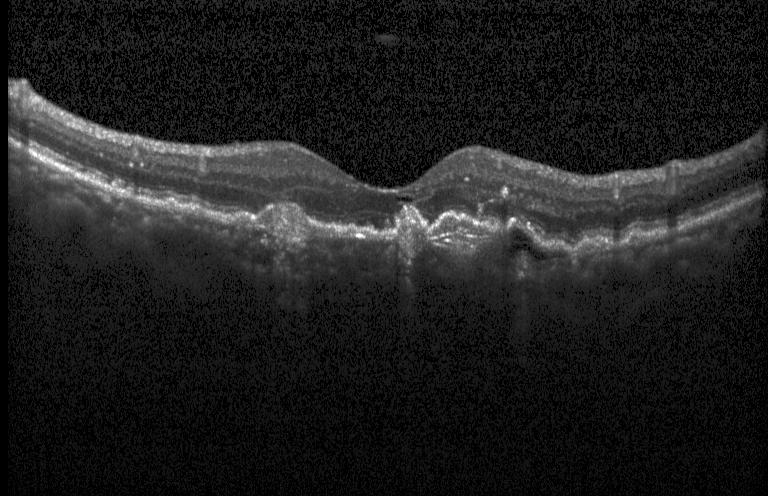

Macular scan; retinal OCT B-scan; spectral-domain optical coherence tomography; instrument: Heidelberg Spectralis. Dx: a choroidal neovascular membrane.